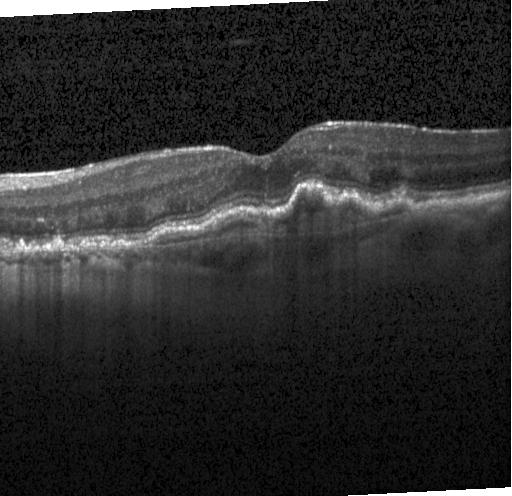 Acquired on a Heidelberg Spectralis. Optical coherence tomography B-scan. Fovea-centered. Spectral-domain OCT. OCT finding: a choroidal neovascular membrane.